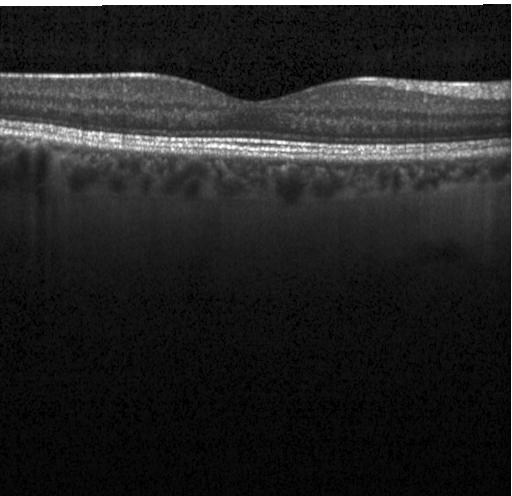 Optical coherence tomography scan
Dx: neither CNV, DME, nor drusen.